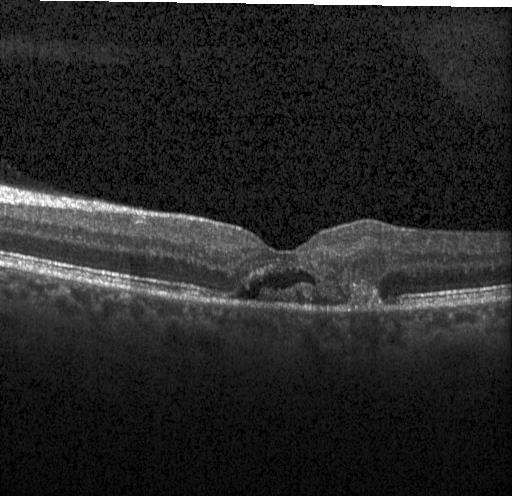
Optical coherence tomography scan
Impression: choroidal neovascularization.